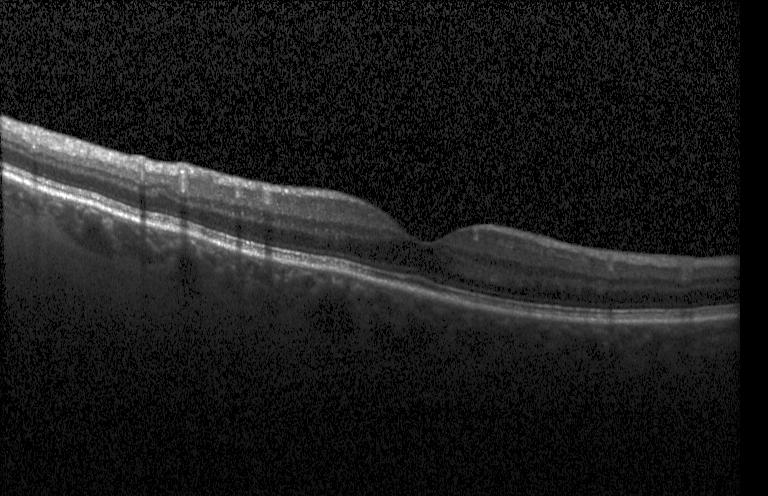

OCT B-scan · instrument: Heidelberg Spectralis — No choroidal neovascularization, no diabetic macular edema, and no drusen.